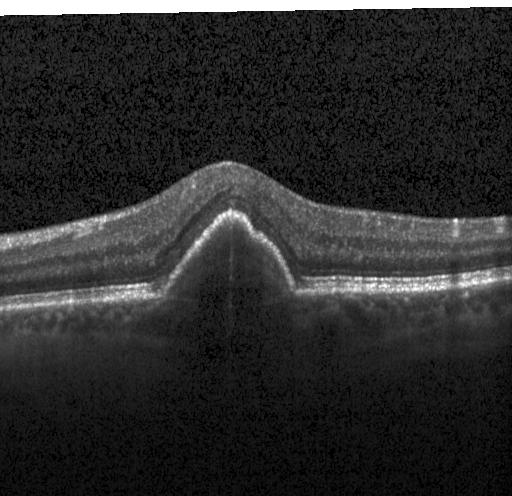 Dx: choroidal neovascularization (CNV).